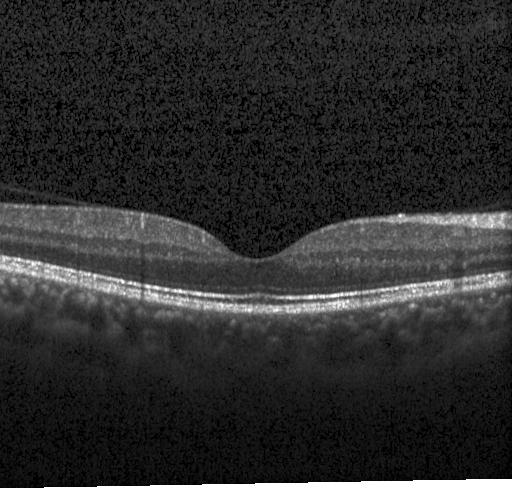 OCT B-scan showing no CNV, DME, or drusen.